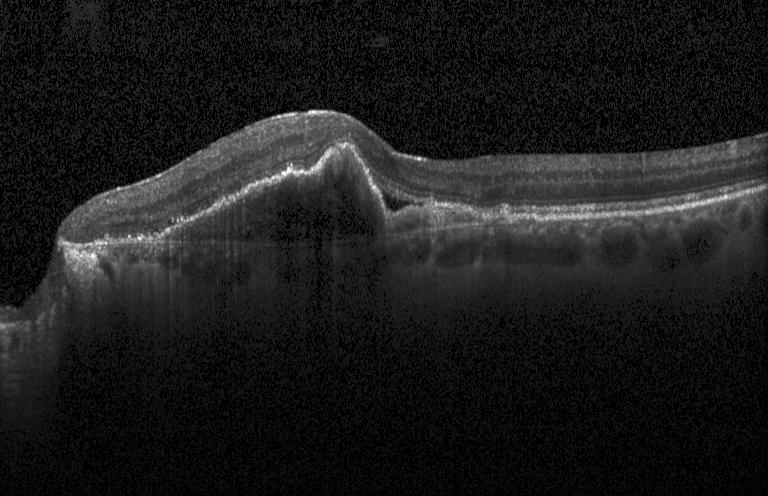 Heidelberg Spectralis OCT system. SD-OCT. Optical coherence tomography scan
Dx: choroidal neovascularization (CNV).